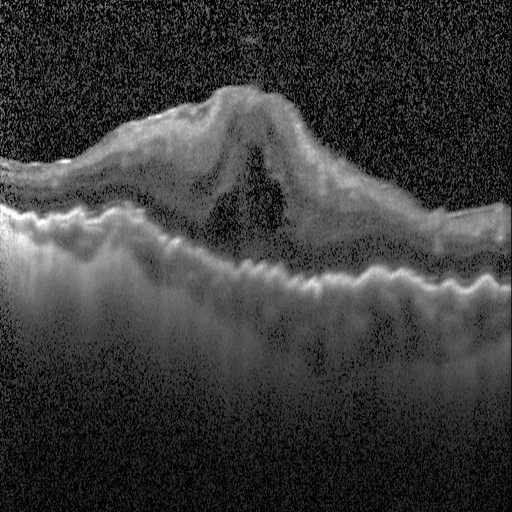
OCT B-scan. Diabetic macular edema.